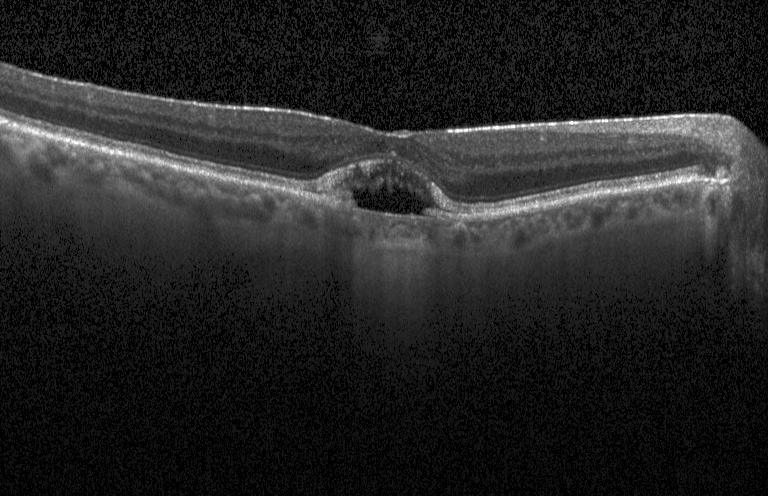
Retinal OCT B-scan · Heidelberg Spectralis · centered on the fovea · spectral-domain optical coherence tomography
Impression: choroidal neovascularization.